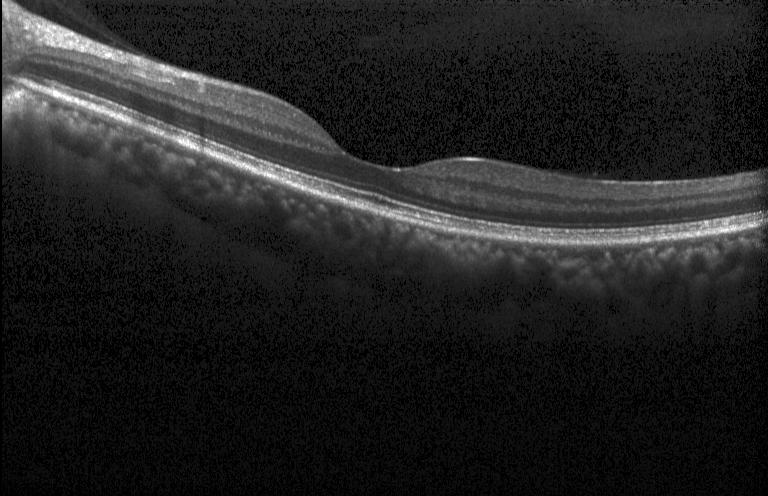
Spectral-domain OCT · OCT line scan.
This B-scan demonstrates no choroidal neovascularization, diabetic macular edema, or drusen.